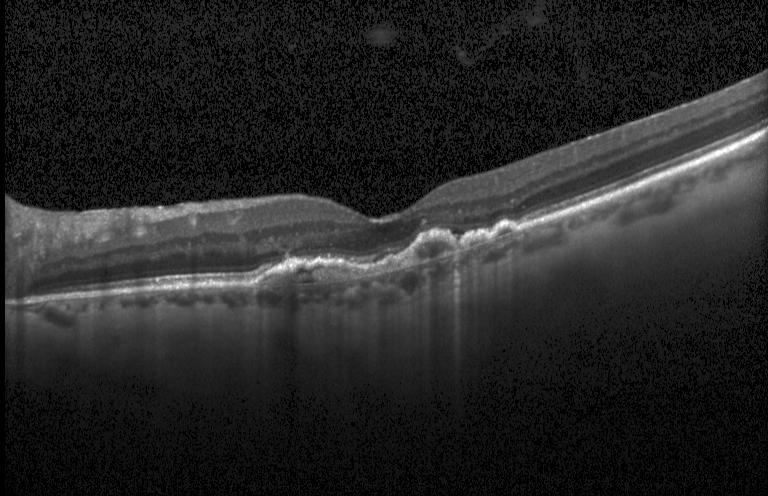

Macular OCT: choroidal neovascularization (CNV).